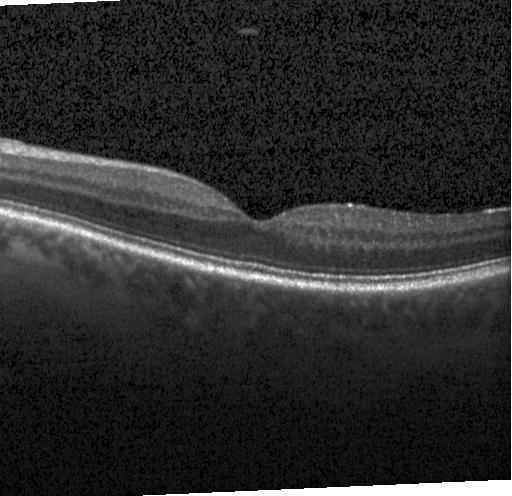 Spectral-domain OCT, OCT line scan, macular scan.
Dx: neither choroidal neovascularization, diabetic macular edema, nor drusen.